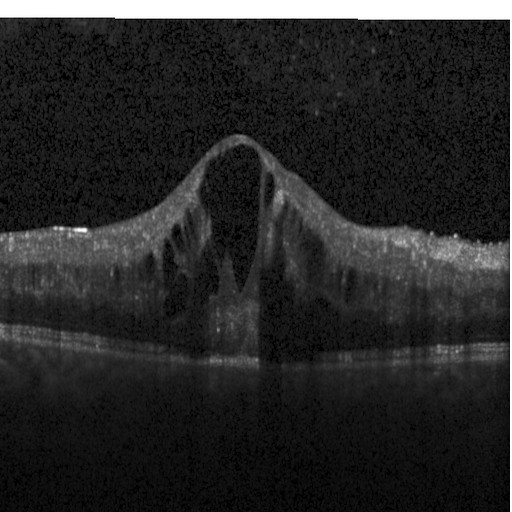 OCT B-scan showing diabetic macular edema.